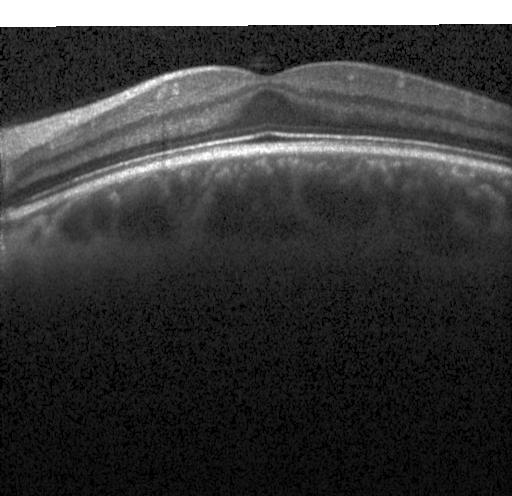 Acquired on a Heidelberg Spectralis. Optical coherence tomography scan.
Impression: no CNV, no DME, and no drusen.